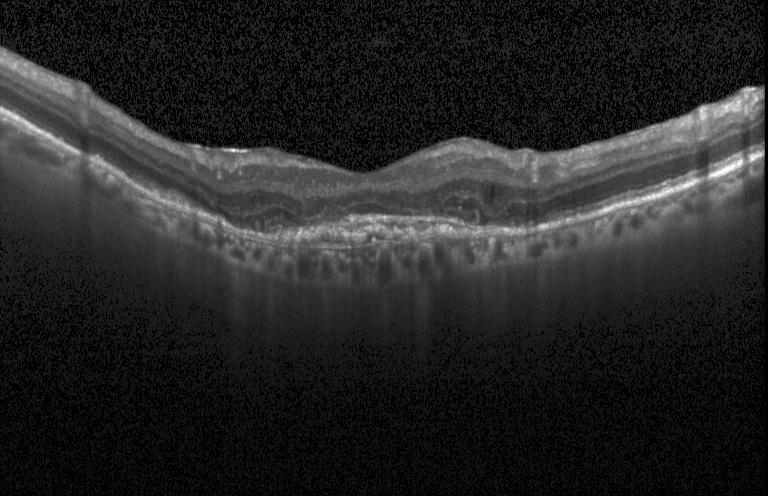

Assessment: a choroidal neovascular membrane.